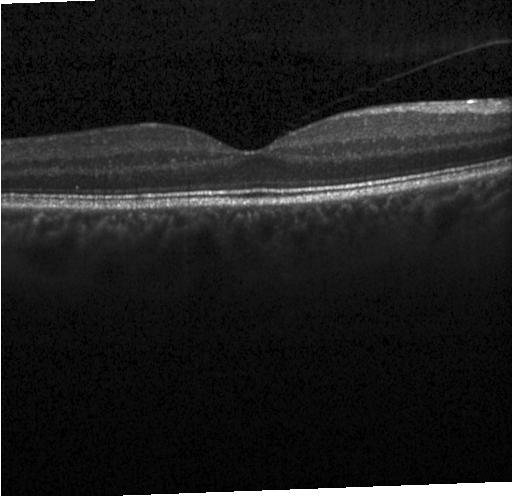

Acquired on a Heidelberg Spectralis · horizontal scan through the fovea · OCT B-scan · spectral-domain optical coherence tomography. Finding: no evidence of CNV, DME, or drusen.